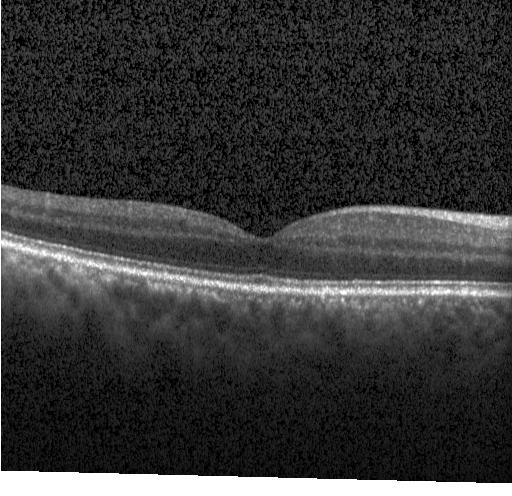 OCT finding: no choroidal neovascularization, diabetic macular edema, or drusen.